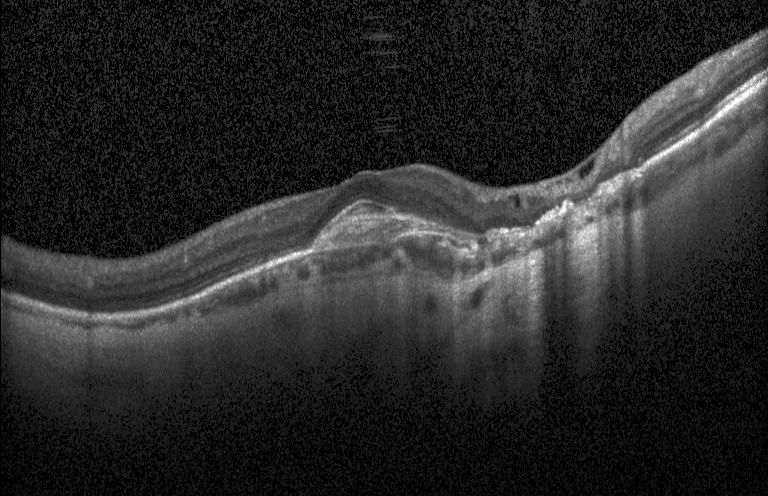 The scan shows choroidal neovascularization (CNV).